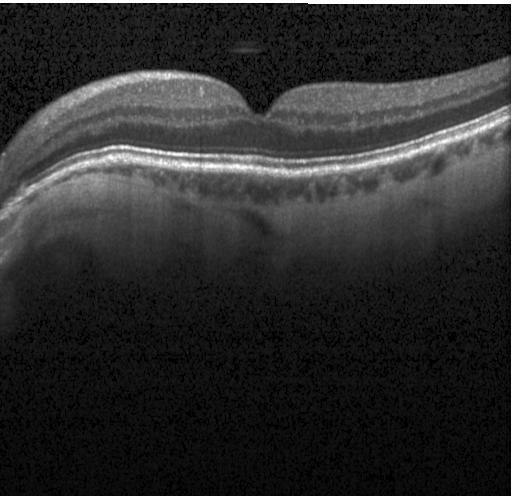

Impression: neither choroidal neovascularization, diabetic macular edema, nor drusen.